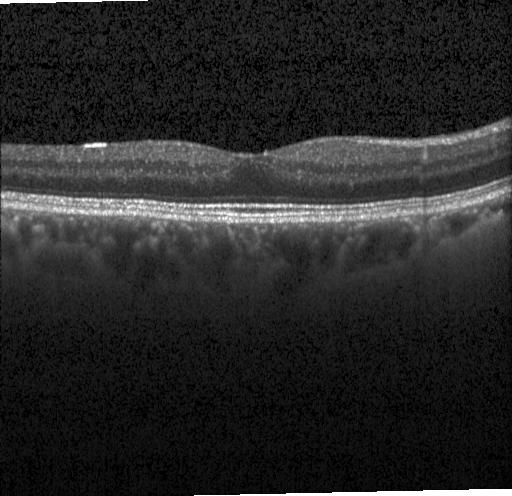 OCT B-scan. SD-OCT. Diagnosis: no CNV, DME, or drusen.